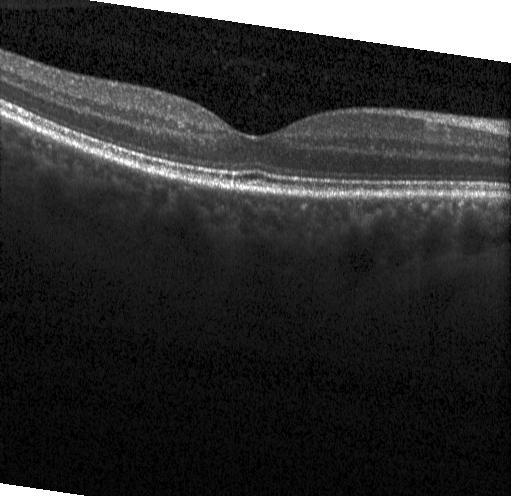 Retinal OCT cross-section. Impression: no CNV, DME, or drusen.